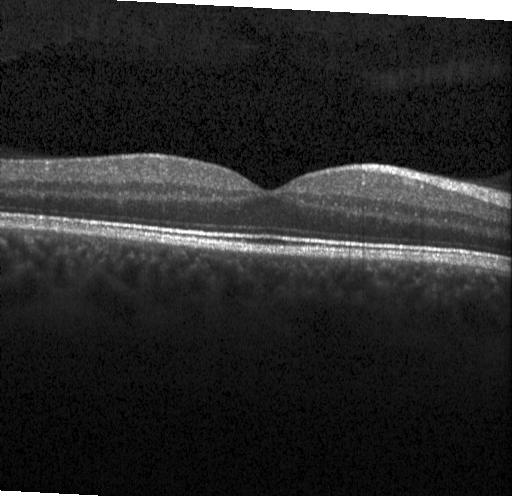

Retinal OCT cross-section showing neither CNV, DME, nor drusen.